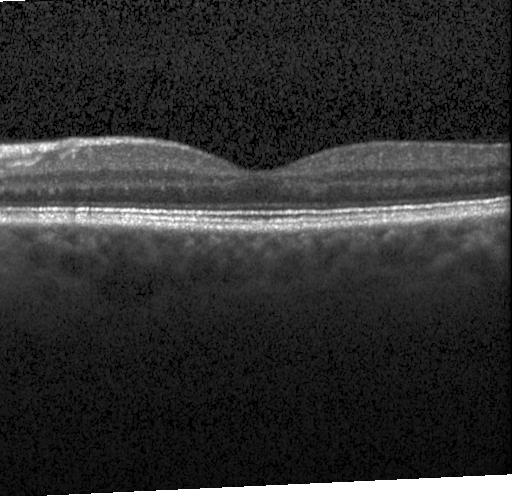

The scan shows no choroidal neovascularization, diabetic macular edema, or drusen.